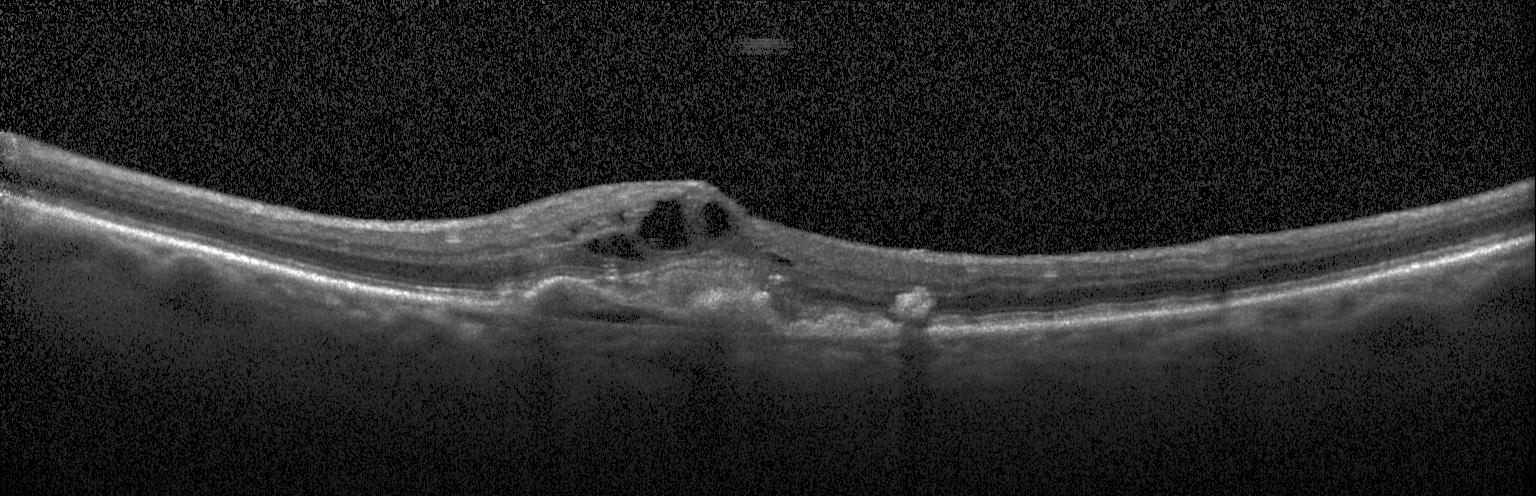

OCT line scan
OCT finding: a choroidal neovascular membrane.